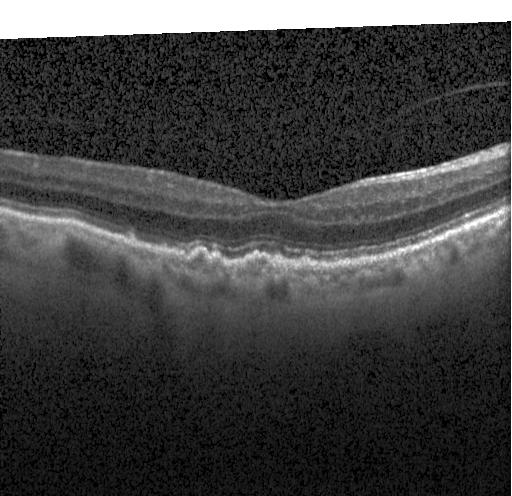
Centered on the fovea, Heidelberg Spectralis OCT system, optical coherence tomography scan, spectral-domain OCT — OCT finding: multiple drusen.